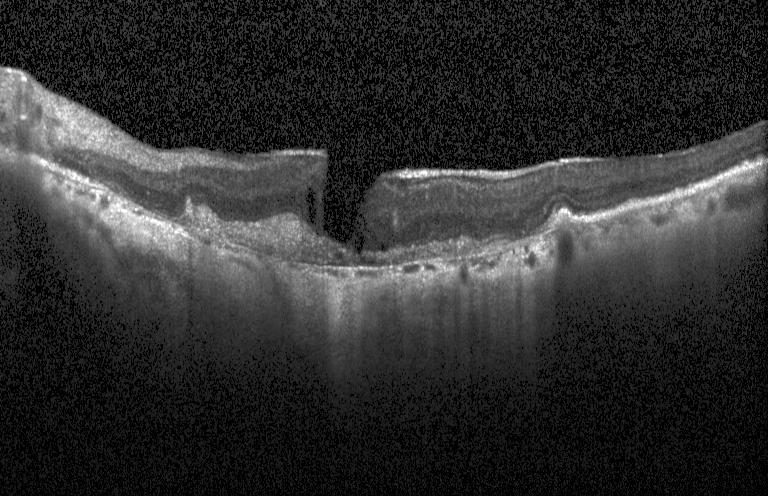 Heidelberg Spectralis OCT system · through the macula · spectral-domain OCT · OCT line scan — Finding: a choroidal neovascular membrane.